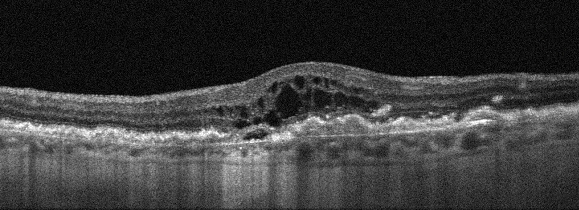
OCT line scan, Optovue Avanti RTVue XR, oculus dexter, fovea-centered. Diagnosis: age-related macular degeneration (AMD).